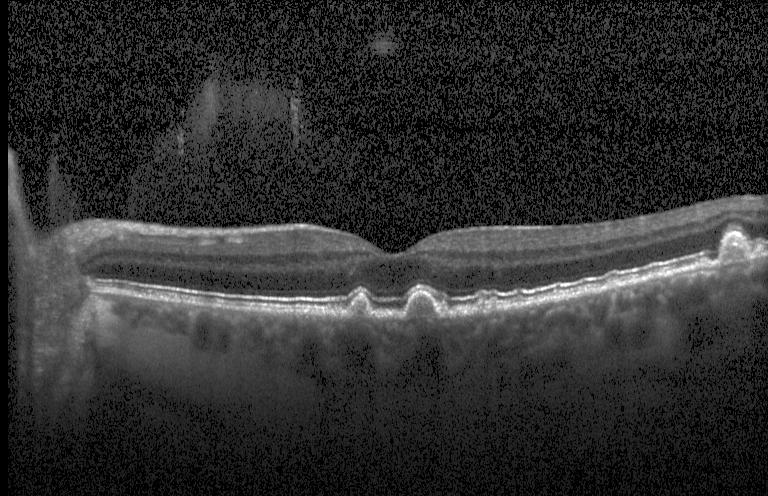

Macular scan, optical coherence tomography B-scan, SD-OCT, acquired on a Heidelberg Spectralis.
Drusen.